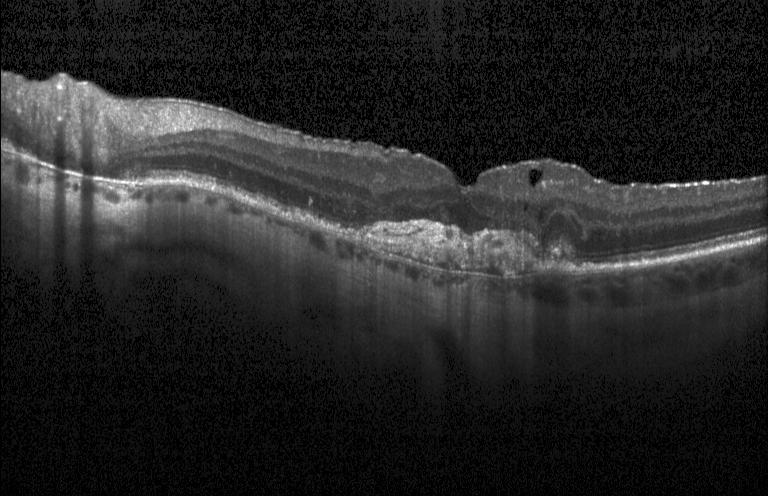 Spectral-domain optical coherence tomography, horizontal scan through the fovea, Heidelberg Spectralis, OCT B-scan. Assessment: choroidal neovascularization (CNV).